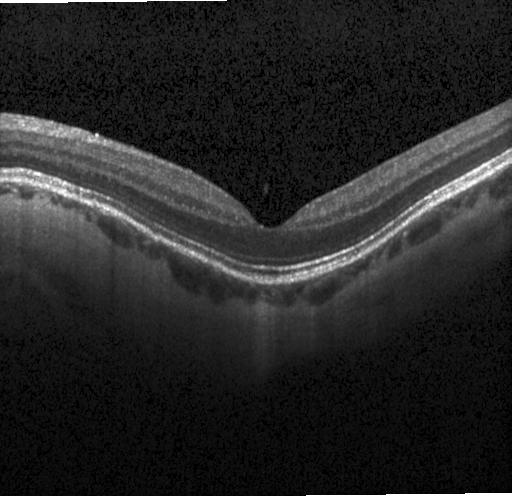 Retinal OCT cross-section, SD-OCT — Diagnosis: no evidence of CNV, DME, or drusen.